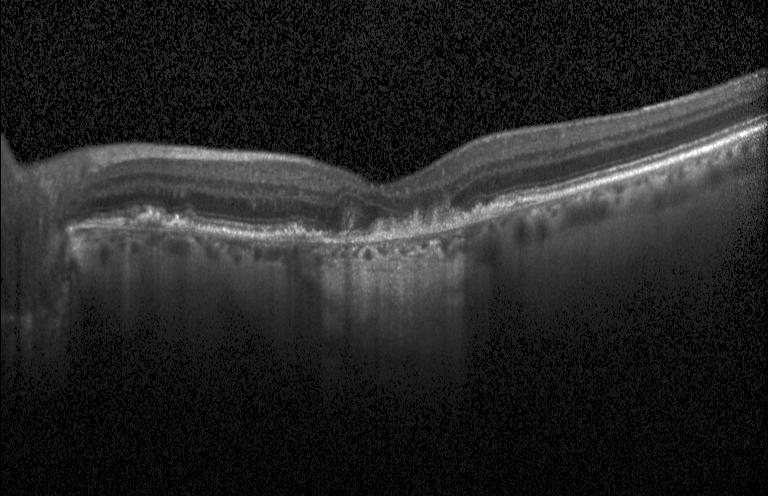

Macular OCT: choroidal neovascularization (CNV).